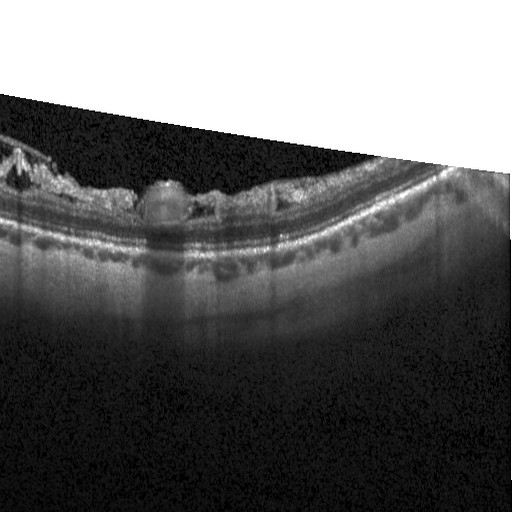

Retinal OCT B-scan. Macular OCT: DME.